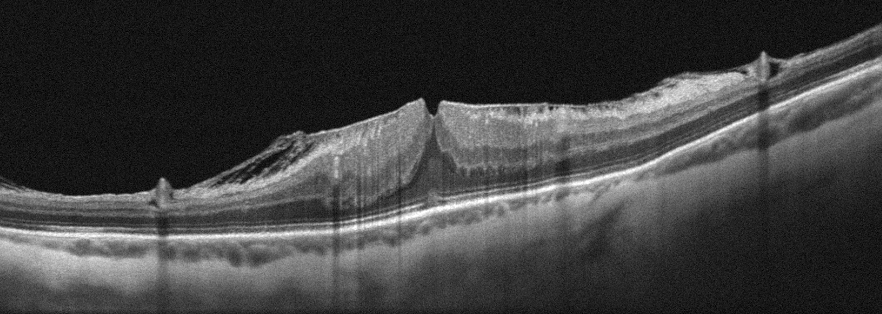

Optical coherence tomography scan · oculus sinister
Dx: ERM.